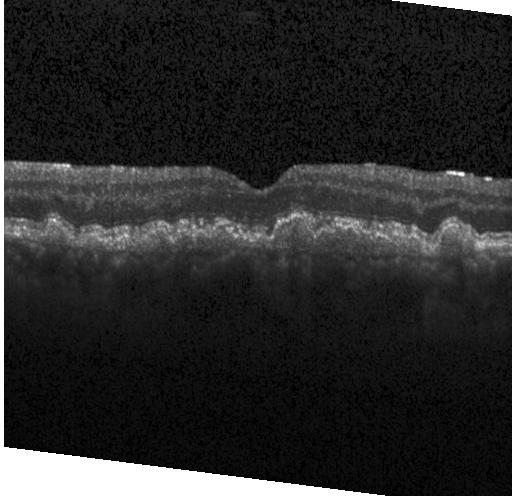 OCT line scan. Finding: CNV.